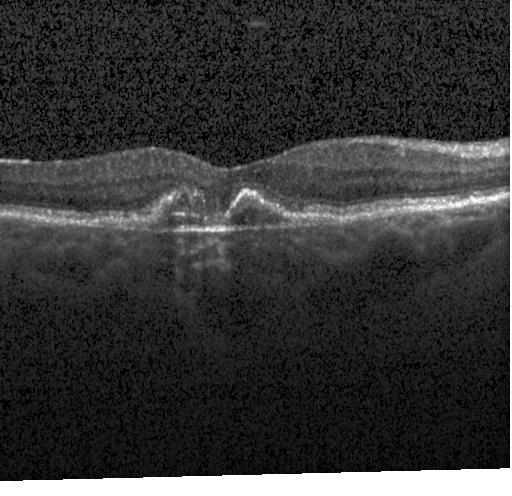

Macular OCT demonstrating a choroidal neovascular membrane.